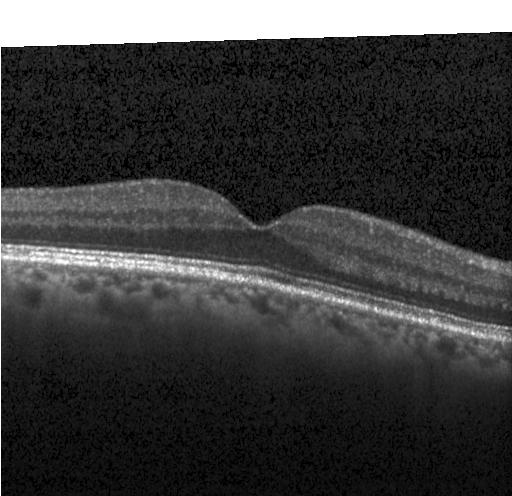 Macular scan · Heidelberg Spectralis OCT system · retinal OCT cross-section.
This B-scan demonstrates neither CNV, DME, nor drusen.